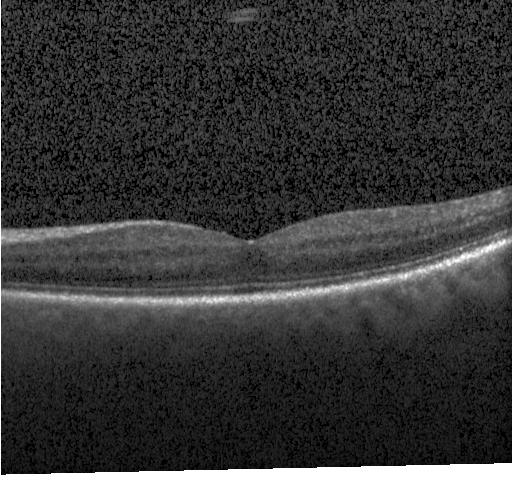

Centered on the fovea, optical coherence tomography B-scan. Finding: no choroidal neovascularization, diabetic macular edema, or drusen.